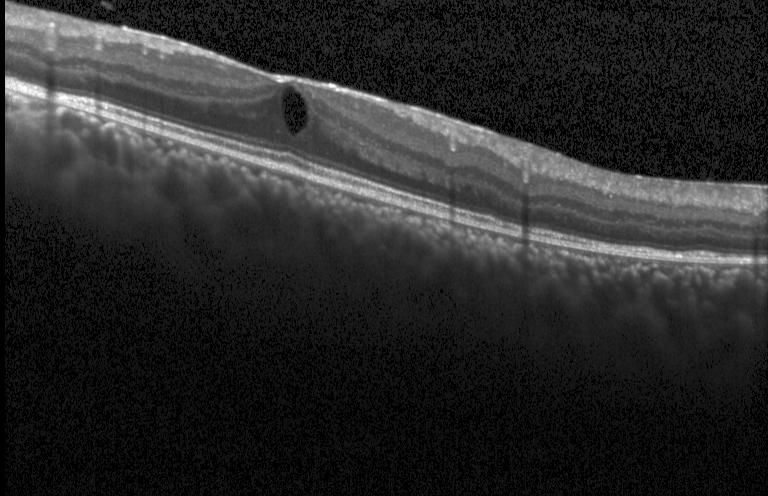 Impression: diabetic macular edema (DME).